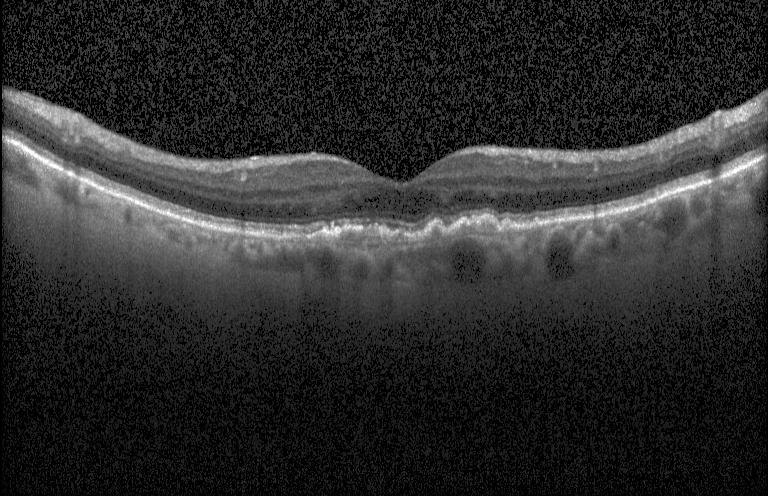

Diagnosis: a choroidal neovascular membrane.